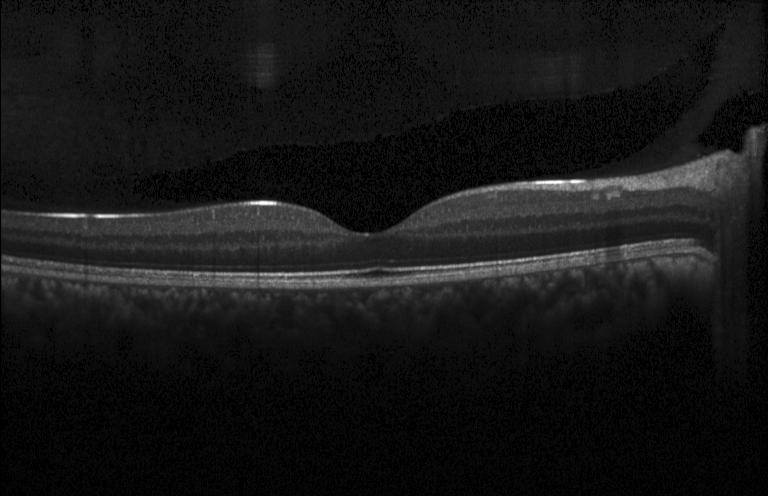
Macular OCT demonstrating no evidence of CNV, DME, or drusen.